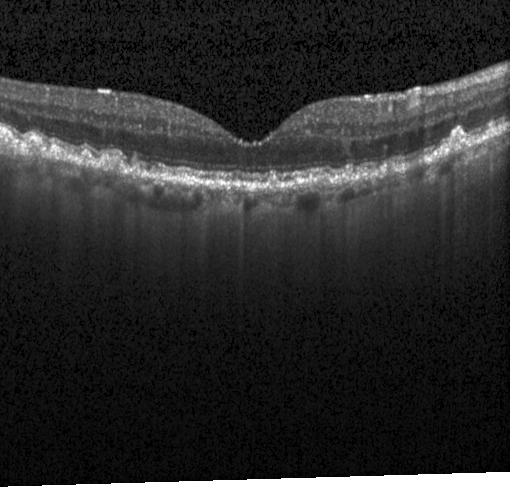 Optical coherence tomography scan, fovea-centered, spectral-domain optical coherence tomography.
Finding: sub-RPE drusenoid deposits.